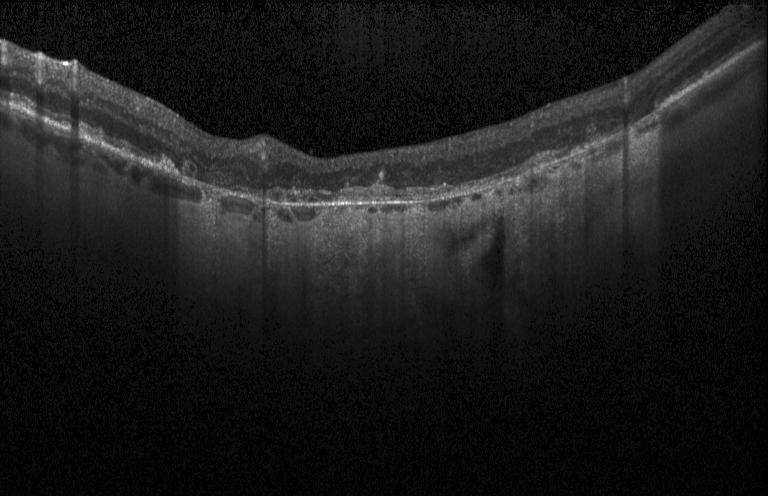
Retinal OCT B-scan, macular scan. OCT finding: a choroidal neovascular membrane.